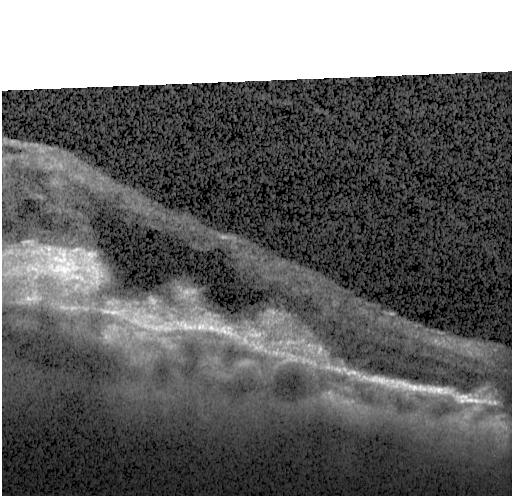
Retinal OCT B-scan.
Assessment: choroidal neovascularization (CNV).